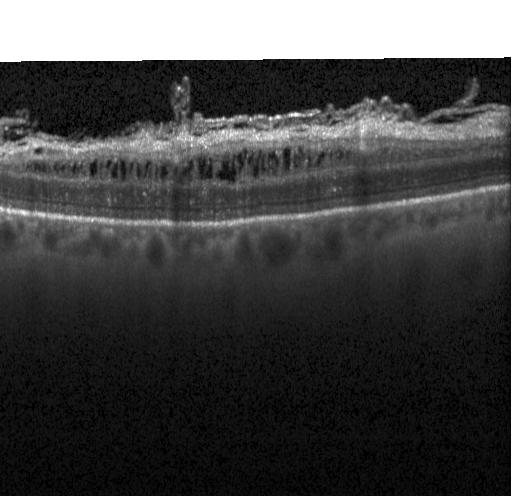
Centered on the fovea · optical coherence tomography scan · Heidelberg Spectralis OCT system. This B-scan demonstrates diabetic macular edema.